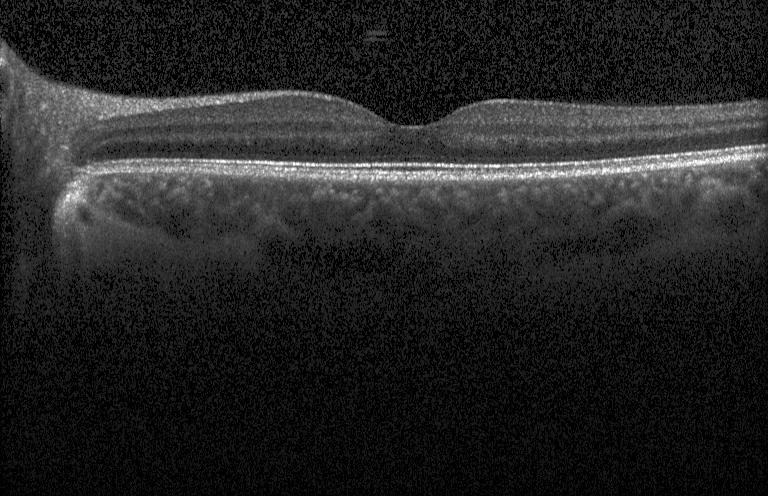
Macular OCT: no evidence of choroidal neovascularization, diabetic macular edema, or drusen.